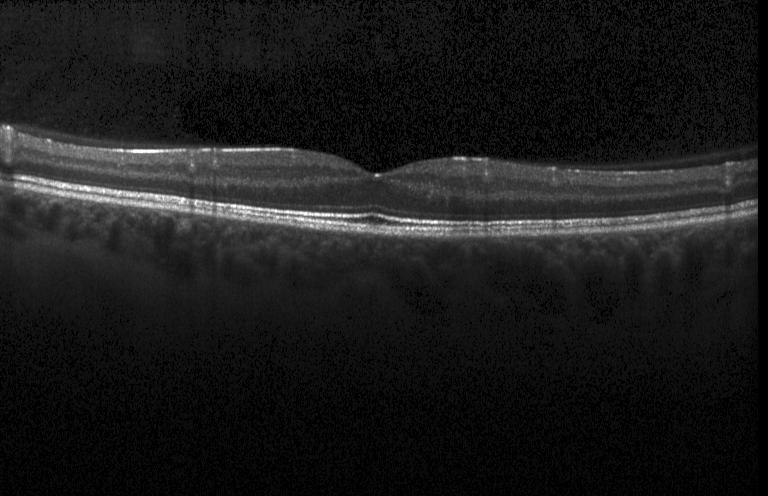
SD-OCT, OCT B-scan
Macular OCT: neither CNV, DME, nor drusen.